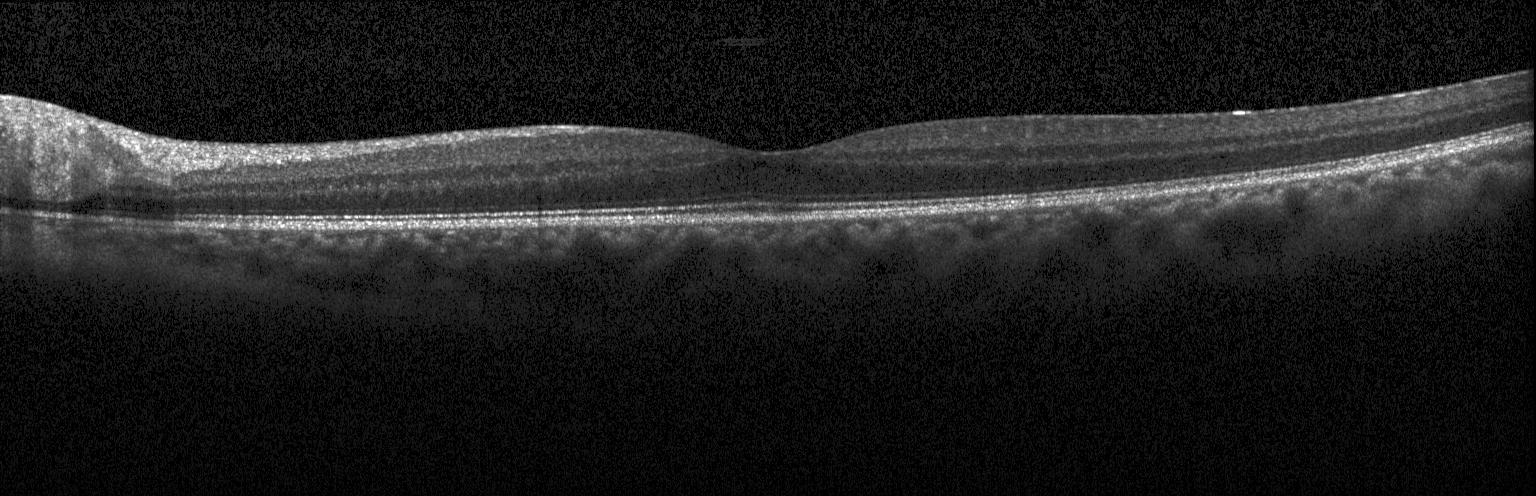
Spectral-domain OCT · OCT B-scan · macular scan. Impression: no choroidal neovascularization, no diabetic macular edema, and no drusen.